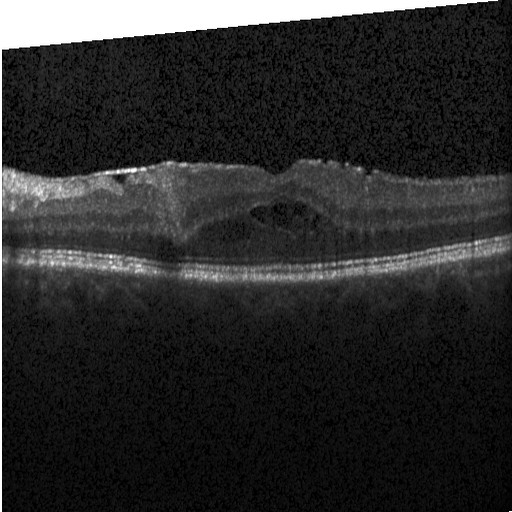
Centered on the fovea. Optical coherence tomography scan. SD-OCT. Acquired on a Heidelberg Spectralis
Assessment: diabetic macular edema.